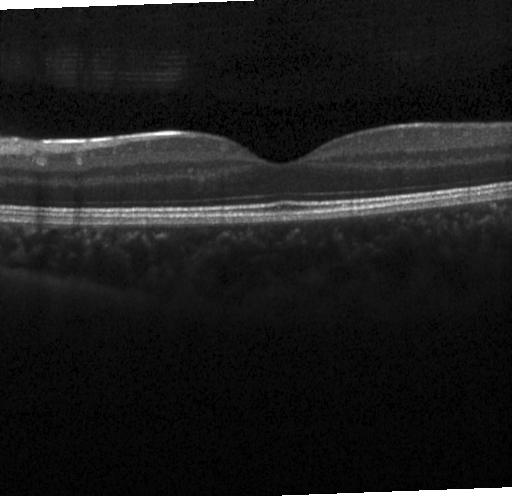
Optical coherence tomography scan.
Impression: no CNV, DME, or drusen.